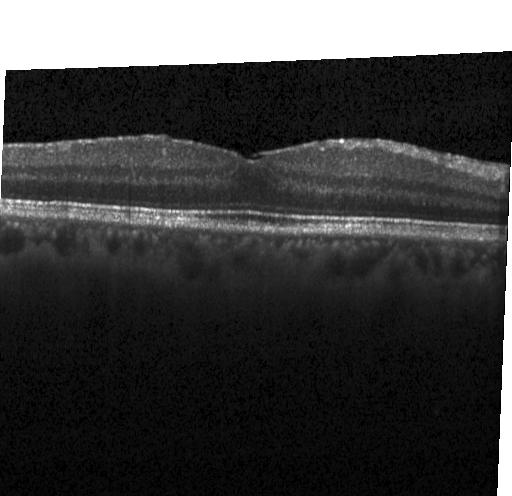 Optical coherence tomography scan; acquired on a Heidelberg Spectralis. Impression: no evidence of CNV, DME, or drusen.